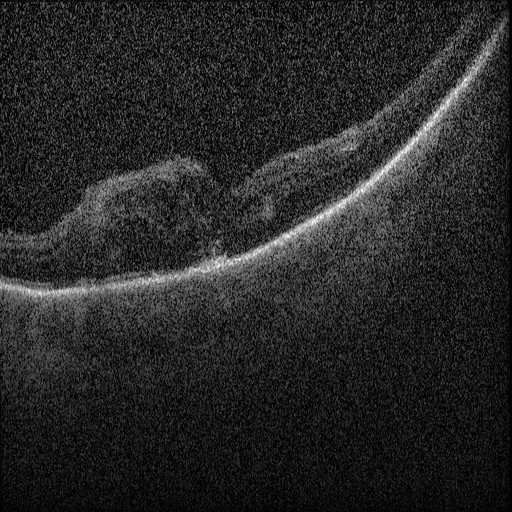
Optical coherence tomography scan — Impression: diabetic macular edema (DME).